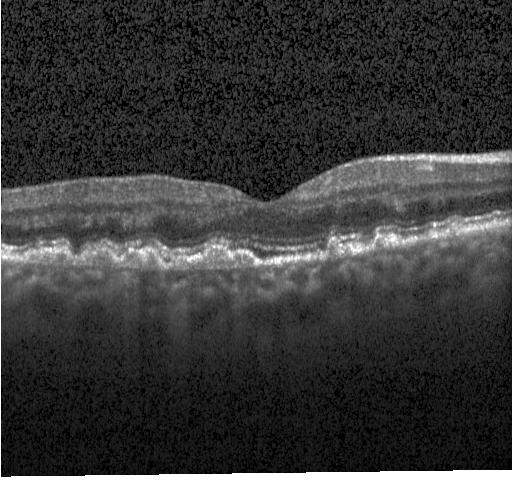
Sub-RPE drusenoid deposits.